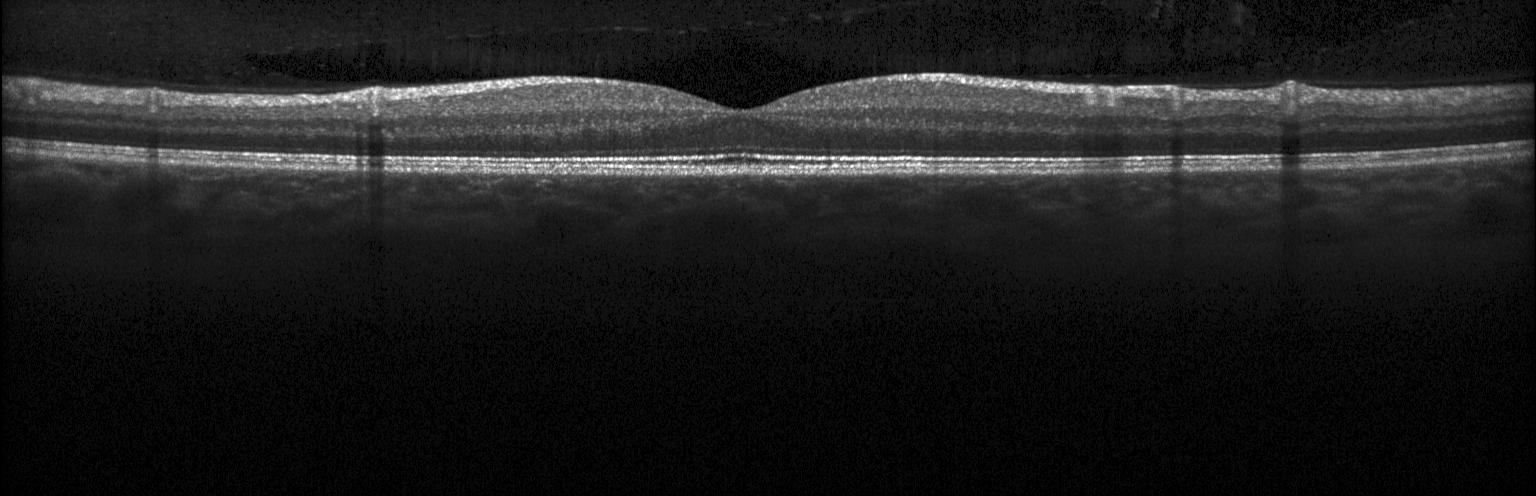

Optical coherence tomography scan
Finding: neither choroidal neovascularization, diabetic macular edema, nor drusen.